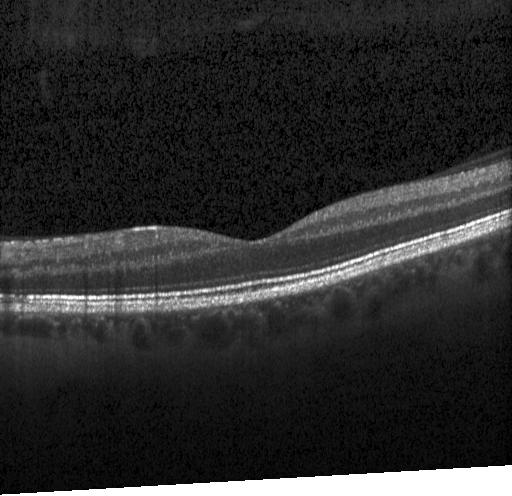 Optical coherence tomography scan.
Impression: no evidence of choroidal neovascularization, diabetic macular edema, or drusen.